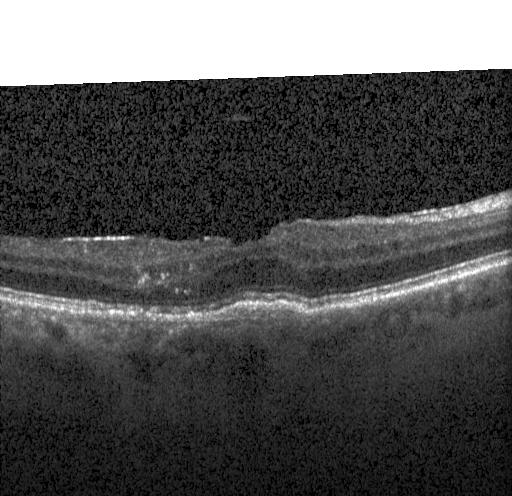
Diagnosis: a choroidal neovascular membrane.